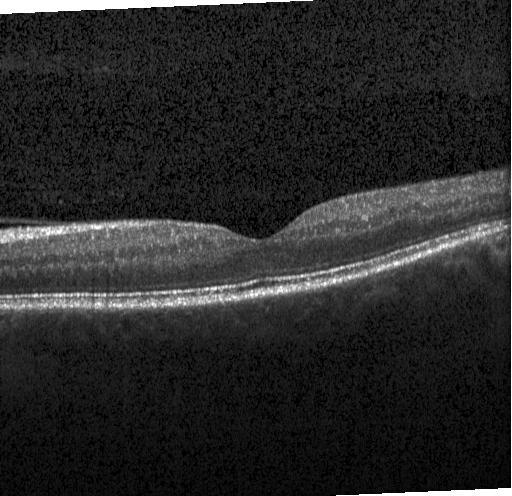

Acquired on a Heidelberg Spectralis, OCT line scan, spectral-domain optical coherence tomography
Neither choroidal neovascularization, diabetic macular edema, nor drusen.